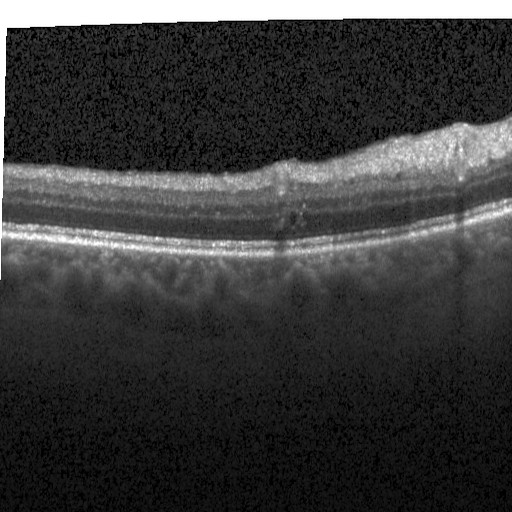

SD-OCT. OCT B-scan. Instrument: Heidelberg Spectralis. Horizontal scan through the fovea — This B-scan demonstrates diabetic macular edema.